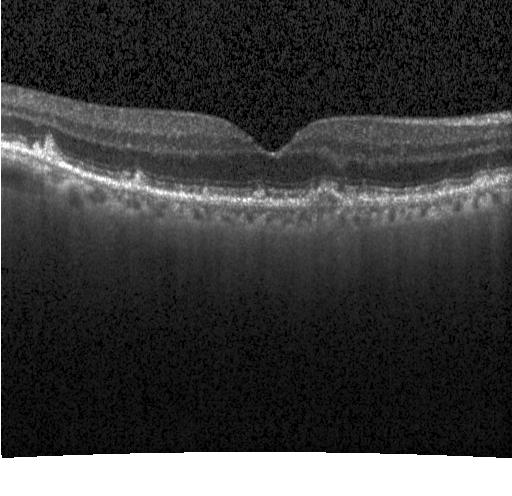

OCT B-scan; spectral-domain optical coherence tomography; Heidelberg Spectralis. Diagnosis: drusen.